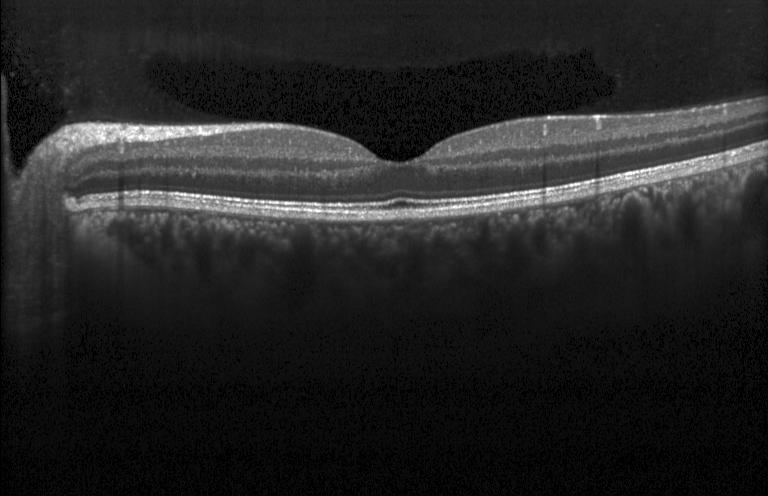 Retinal OCT cross-section; macular scan; Heidelberg Spectralis OCT system; spectral-domain optical coherence tomography.
Finding: no CNV, DME, or drusen.